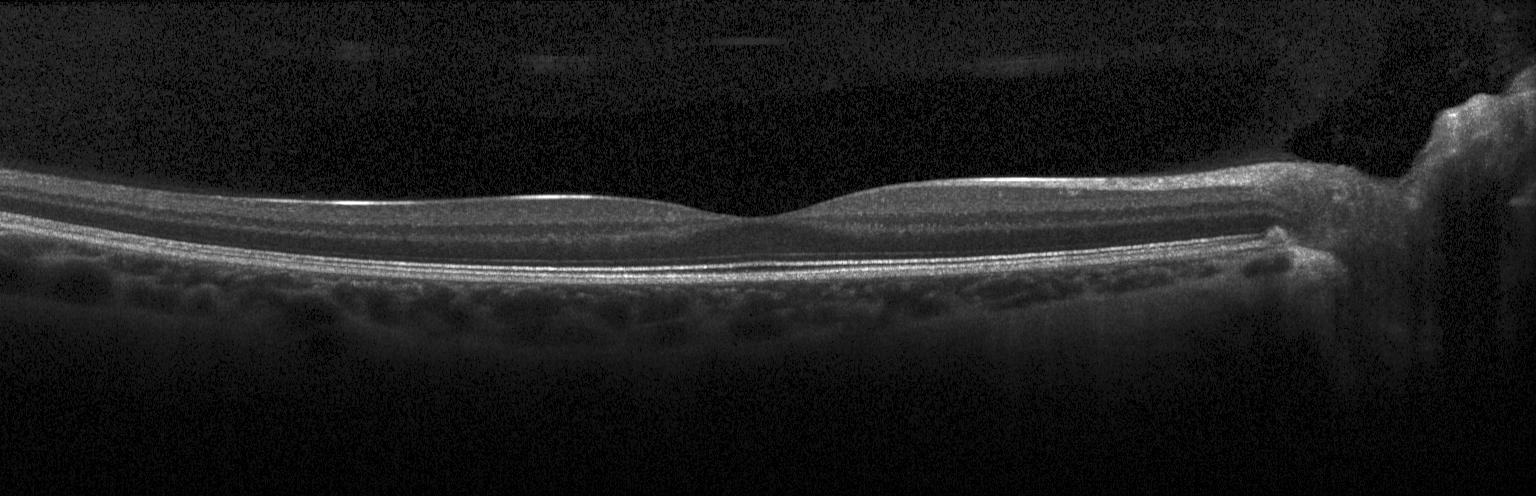
OCT line scan — Finding: no choroidal neovascularization, diabetic macular edema, or drusen.